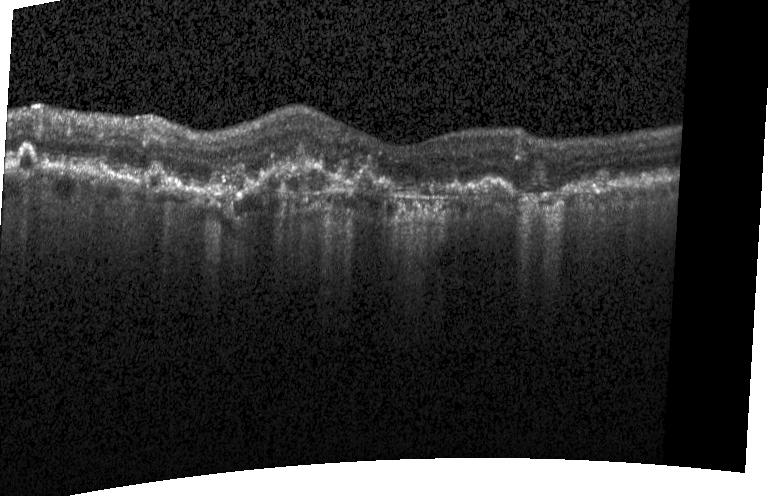

The scan shows CNV.